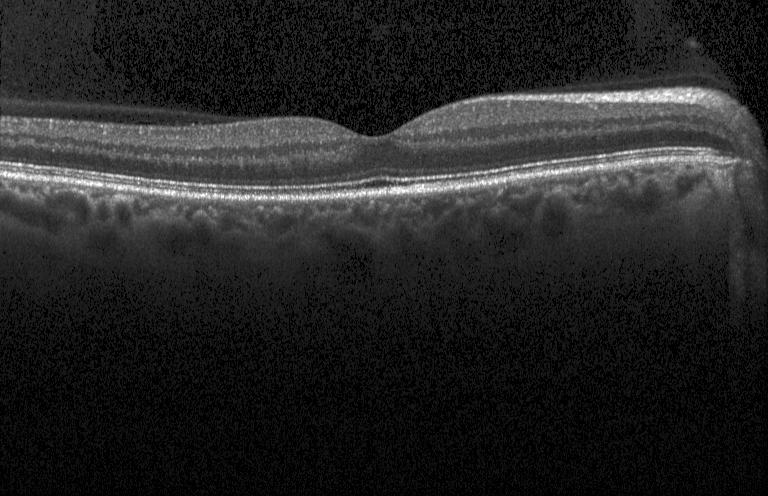
OCT scan showing neither choroidal neovascularization, diabetic macular edema, nor drusen.